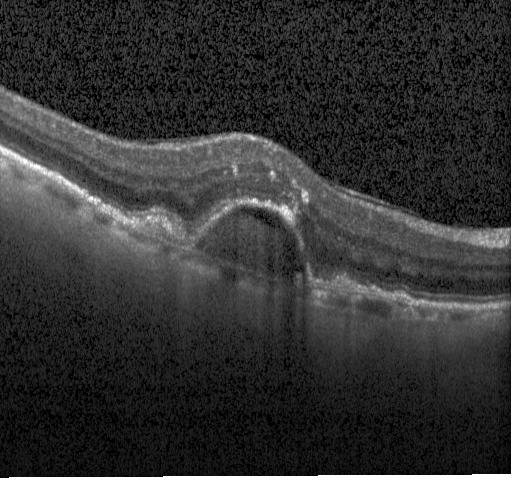
Macular OCT: choroidal neovascularization.